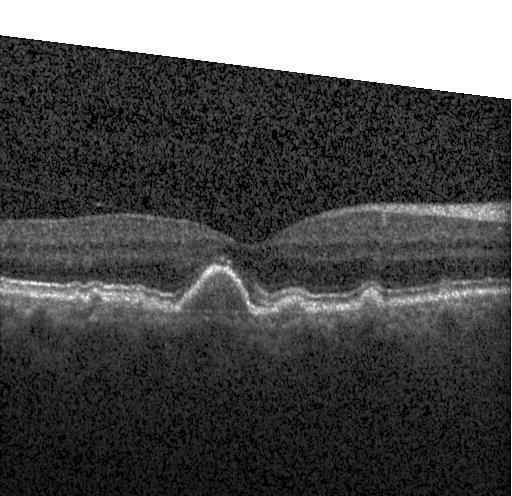 Heidelberg Spectralis OCT system, optical coherence tomography scan. Diagnosis: drusen.